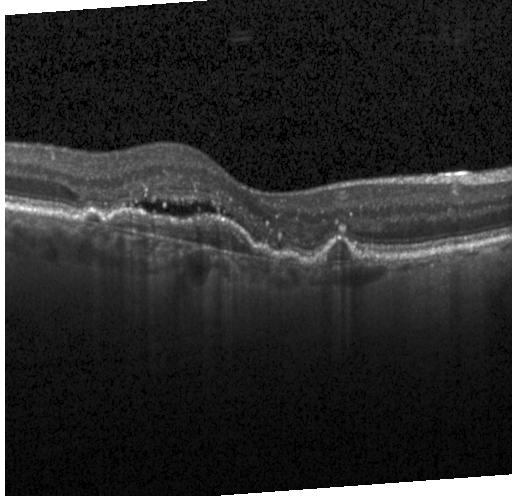
OCT line scan; acquired on a Heidelberg Spectralis; SD-OCT
Choroidal neovascularization.